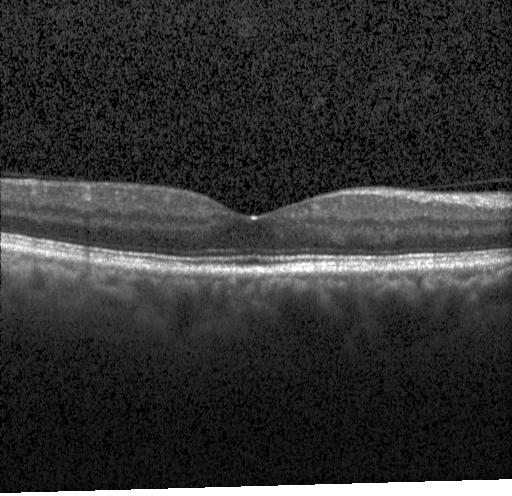 Retinal OCT cross-section, acquired on a Heidelberg Spectralis — Neither choroidal neovascularization, diabetic macular edema, nor drusen.